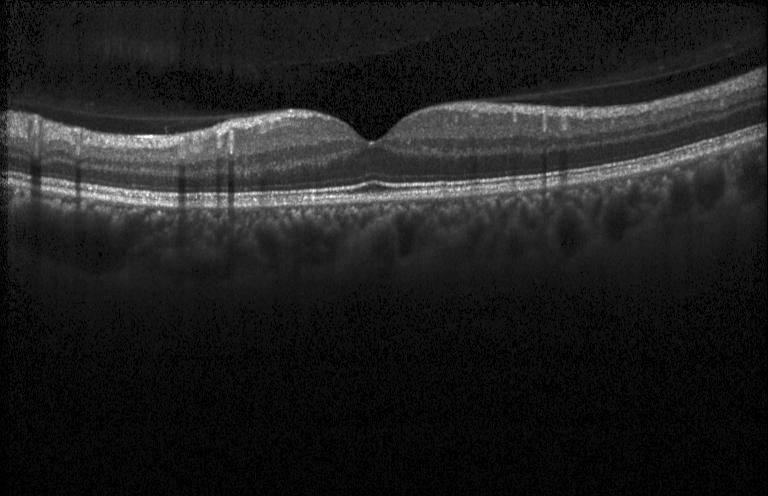

Heidelberg Spectralis, OCT line scan, macular scan, spectral-domain optical coherence tomography — No choroidal neovascularization, diabetic macular edema, or drusen.